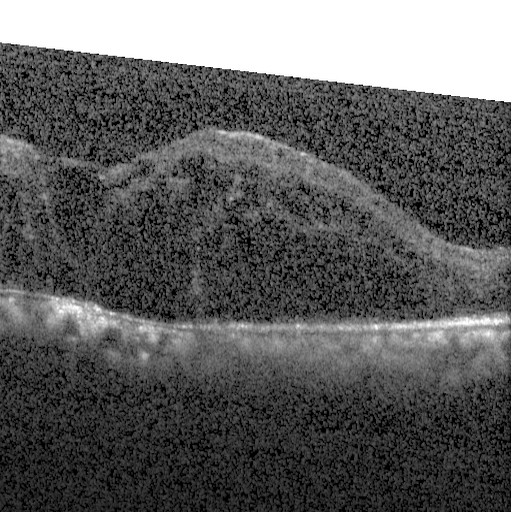
Acquired on a Heidelberg Spectralis · OCT B-scan · fovea-centered · spectral-domain optical coherence tomography.
This B-scan demonstrates DME.